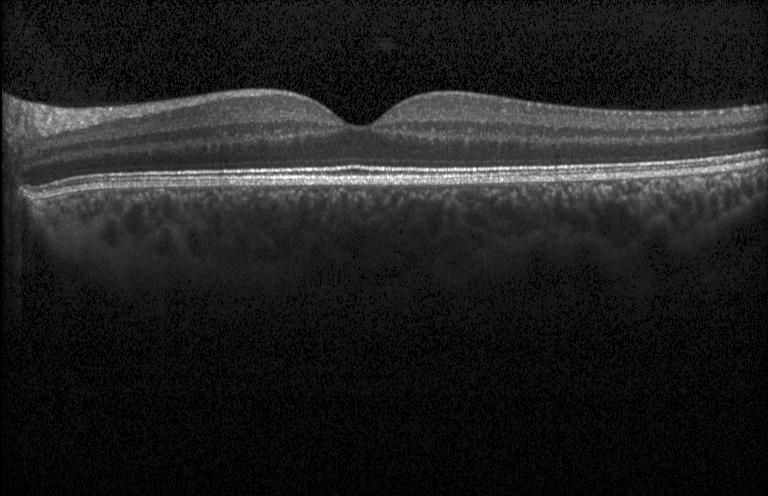

OCT line scan
Assessment: no evidence of choroidal neovascularization, diabetic macular edema, or drusen.